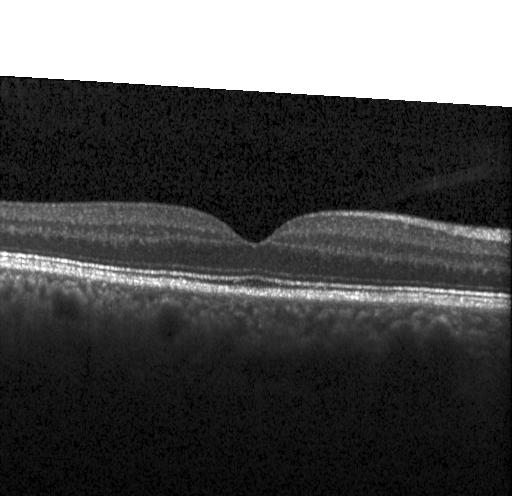 OCT finding: no CNV, DME, or drusen.